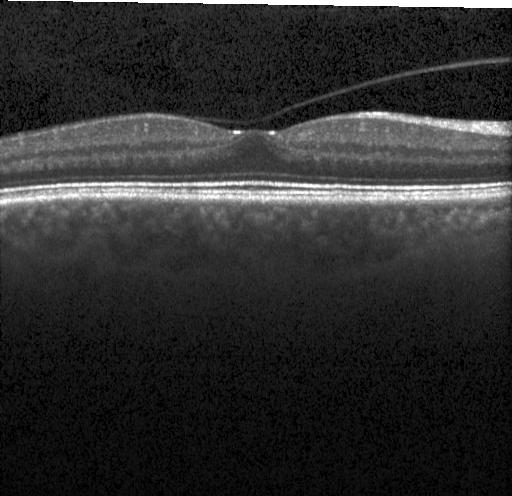
Neither choroidal neovascularization, diabetic macular edema, nor drusen.